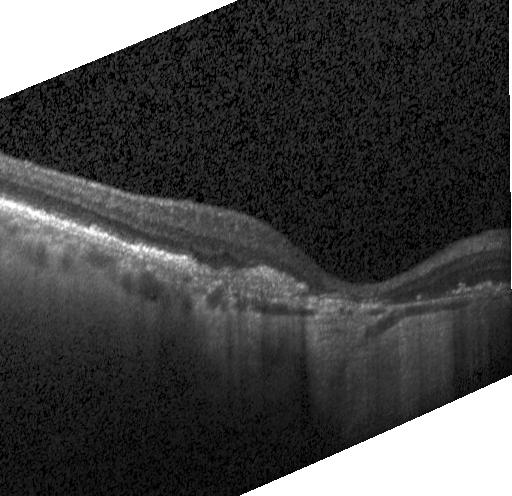
Through the macula, Heidelberg Spectralis, retinal OCT cross-section
Dx: a choroidal neovascular membrane.